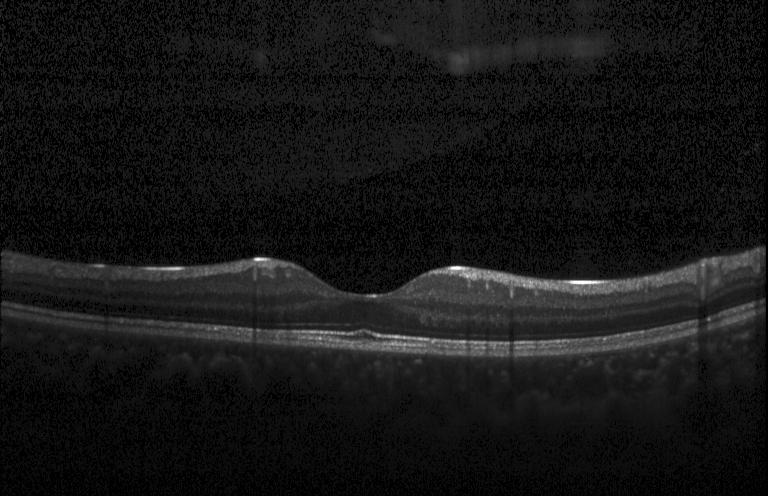 Optical coherence tomography B-scan, through the macula, Heidelberg Spectralis, spectral-domain optical coherence tomography — Diagnosis: no choroidal neovascularization, no diabetic macular edema, and no drusen.